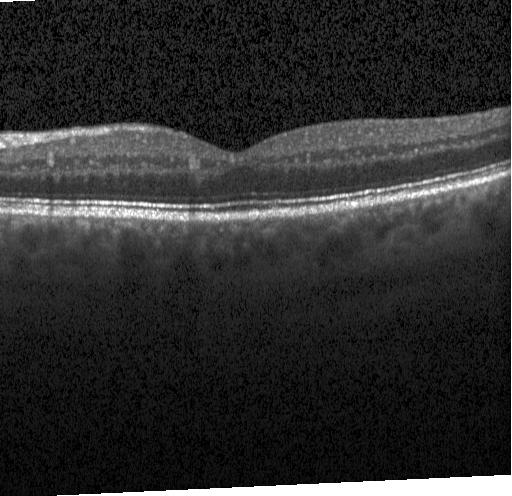 Centered on the fovea; Heidelberg Spectralis; optical coherence tomography scan.
Dx: no CNV, no DME, and no drusen.